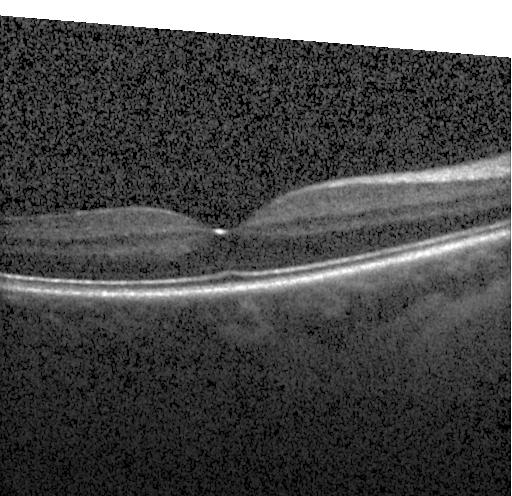 Finding: neither choroidal neovascularization, diabetic macular edema, nor drusen.